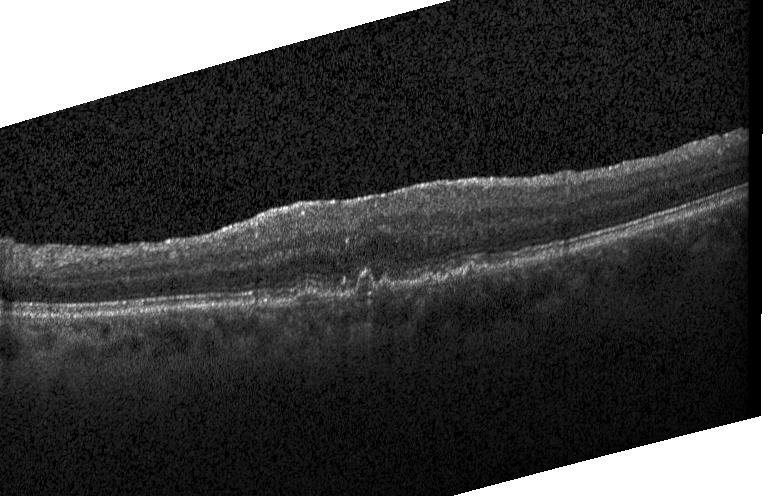
Retinal OCT B-scan; Heidelberg Spectralis OCT system — Dx: drusen.